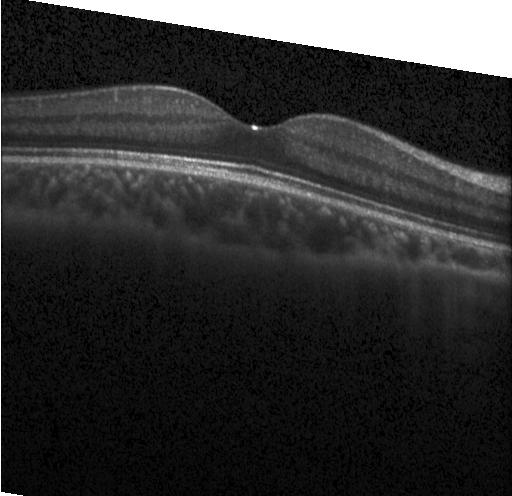

Finding: no evidence of choroidal neovascularization, diabetic macular edema, or drusen.